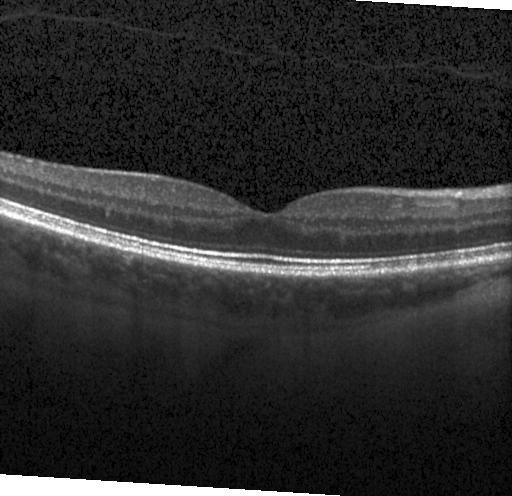

Instrument: Heidelberg Spectralis; OCT B-scan
Finding: neither choroidal neovascularization, diabetic macular edema, nor drusen.